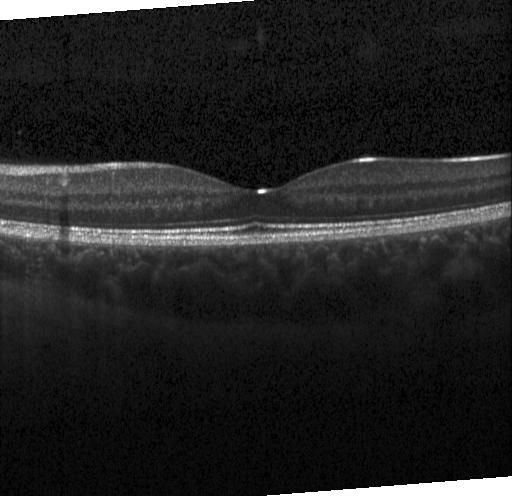 This B-scan demonstrates no choroidal neovascularization, no diabetic macular edema, and no drusen.